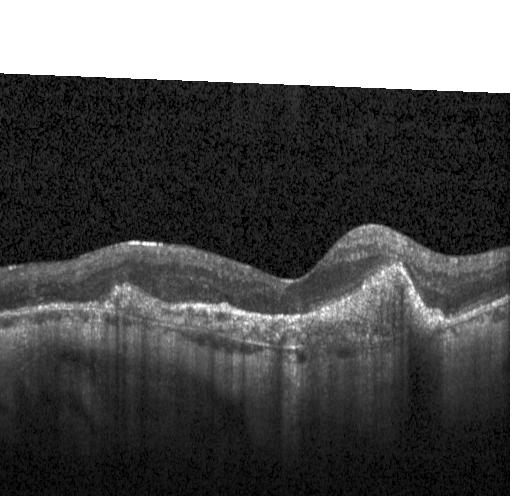

SD-OCT · macular scan · OCT line scan
CNV.